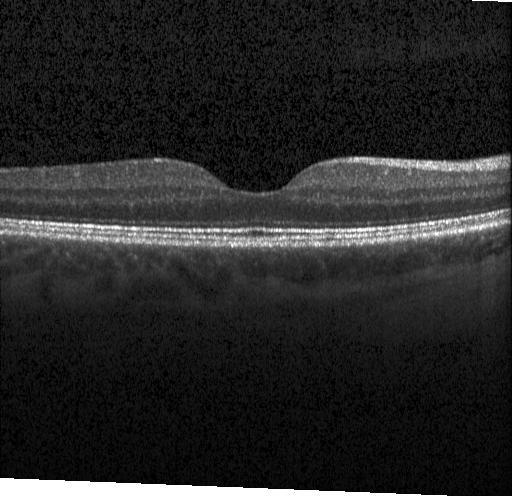
Fovea-centered, retinal OCT B-scan, acquired on a Heidelberg Spectralis — This B-scan demonstrates no evidence of CNV, DME, or drusen.